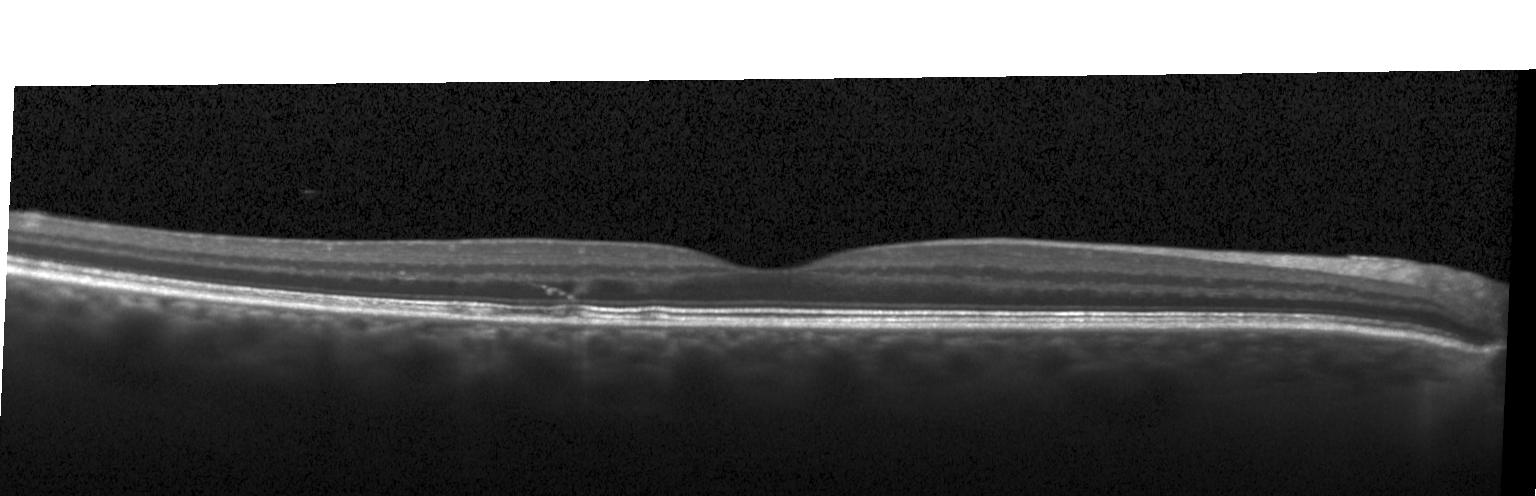

This B-scan demonstrates no CNV, DME, or drusen.